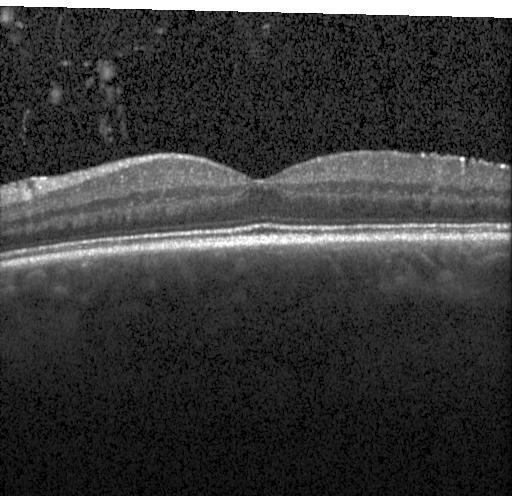 Optical coherence tomography scan; macular scan; Heidelberg Spectralis; spectral-domain optical coherence tomography. No CNV, no DME, and no drusen.